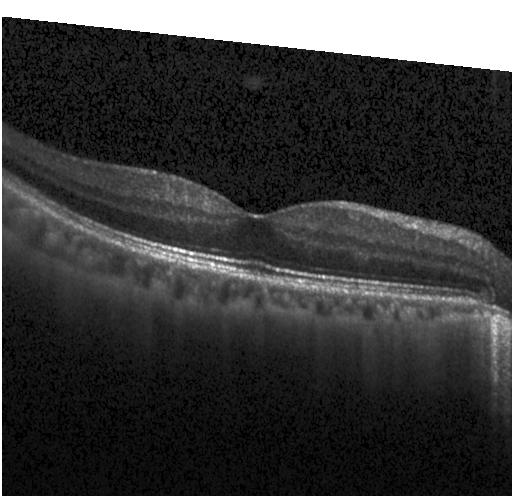

Assessment: neither CNV, DME, nor drusen.